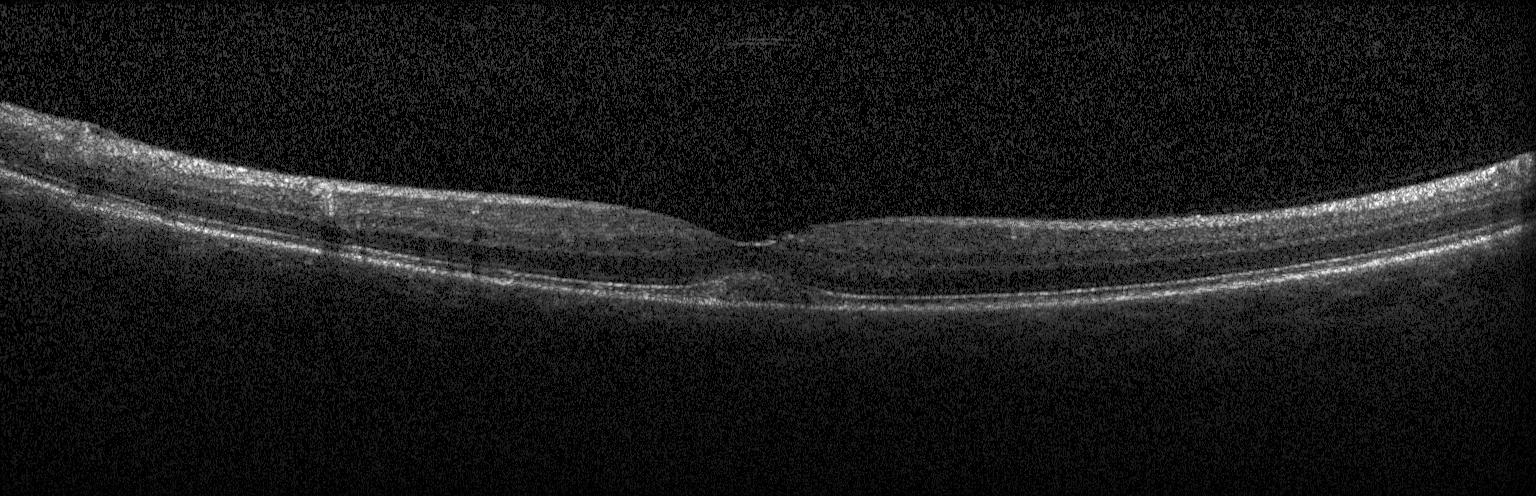
Macular OCT: choroidal neovascularization.